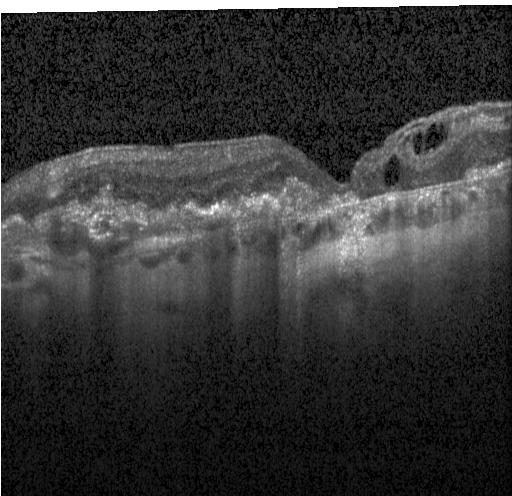
Instrument: Heidelberg Spectralis · SD-OCT · retinal OCT cross-section — Finding: choroidal neovascularization.